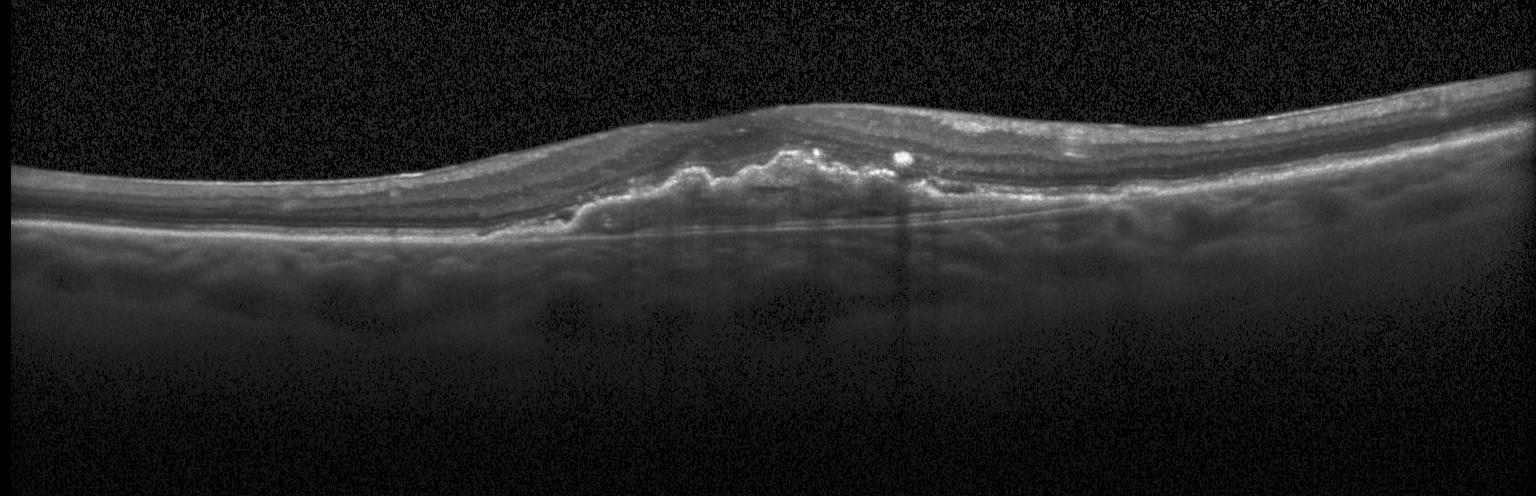

Heidelberg Spectralis OCT system. Centered on the fovea. OCT line scan.
Assessment: choroidal neovascularization (CNV).